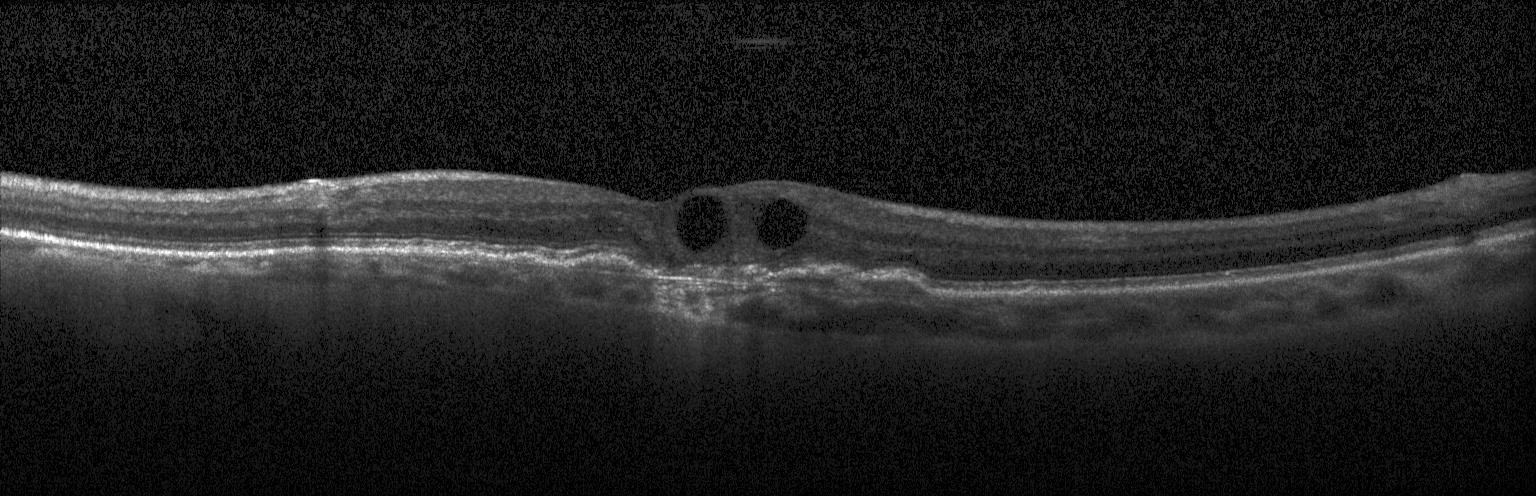

Macular OCT: choroidal neovascularization.